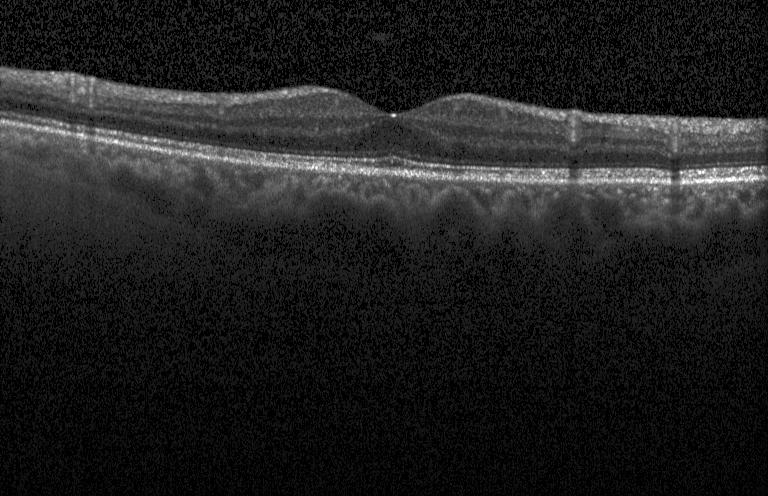
Retinal OCT cross-section showing no evidence of choroidal neovascularization, diabetic macular edema, or drusen.